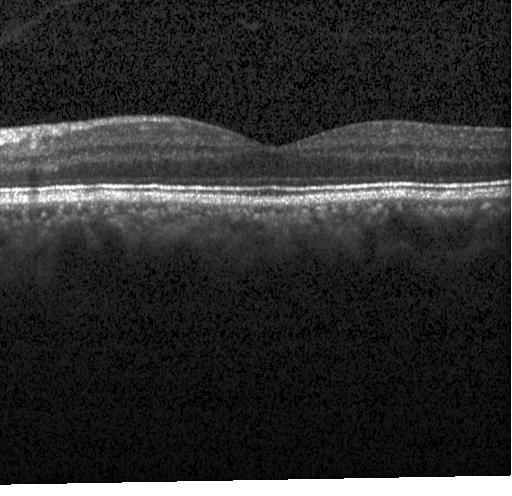

The scan shows no choroidal neovascularization, diabetic macular edema, or drusen.